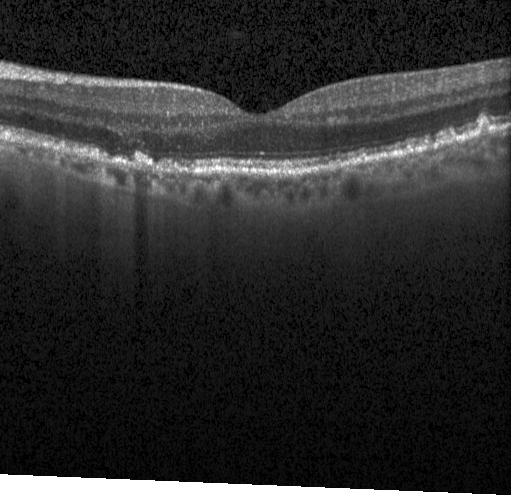 OCT B-scan, horizontal scan through the fovea. Impression: drusen.